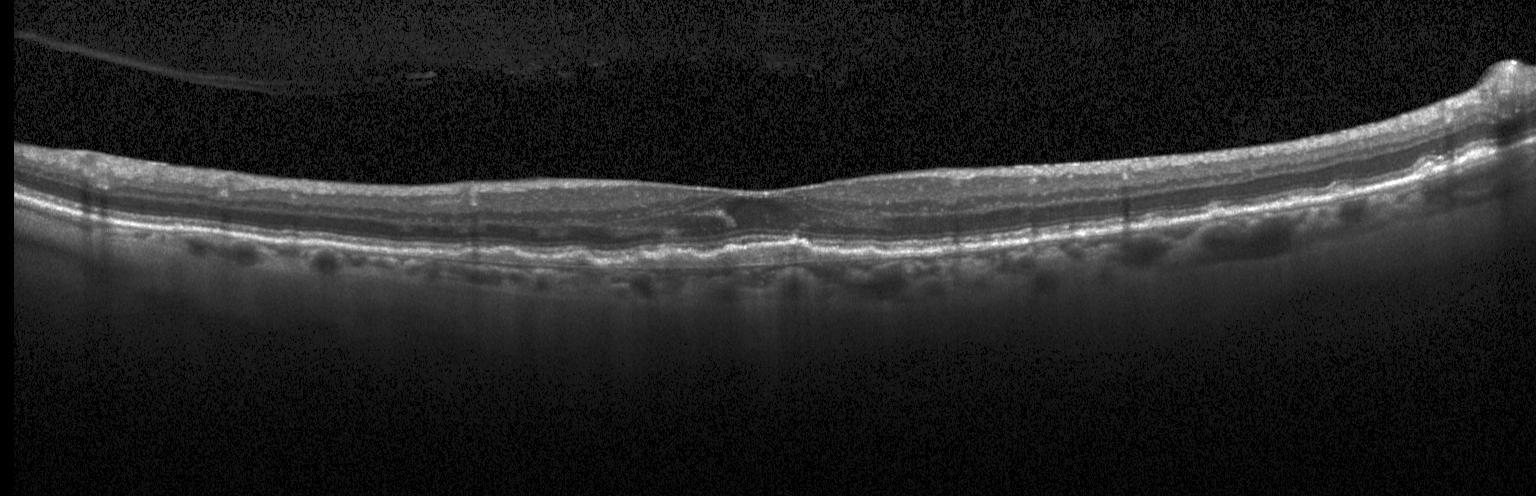 Optical coherence tomography B-scan.
OCT finding: choroidal neovascularization.